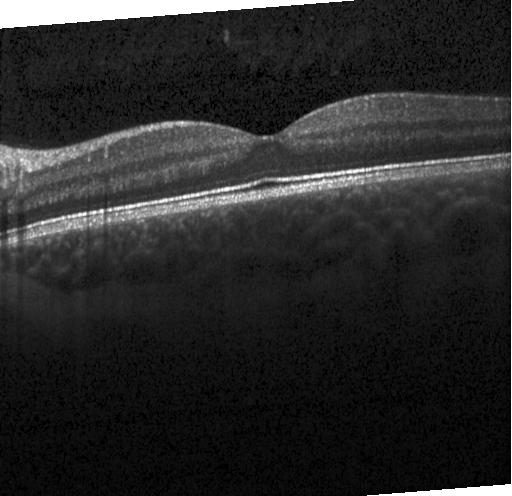
Fovea-centered · Heidelberg Spectralis · OCT B-scan. Impression: no CNV, no DME, and no drusen.